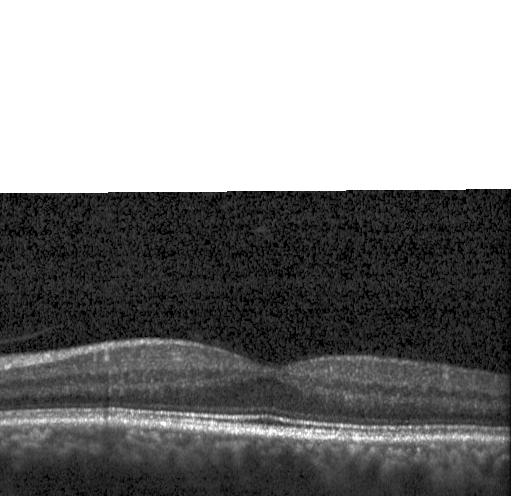
Spectral-domain OCT B-scan: no choroidal neovascularization, no diabetic macular edema, and no drusen.